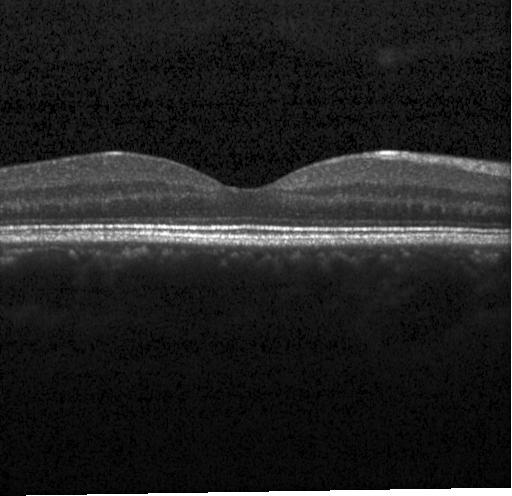

Optical coherence tomography scan — Assessment: no choroidal neovascularization, no diabetic macular edema, and no drusen.